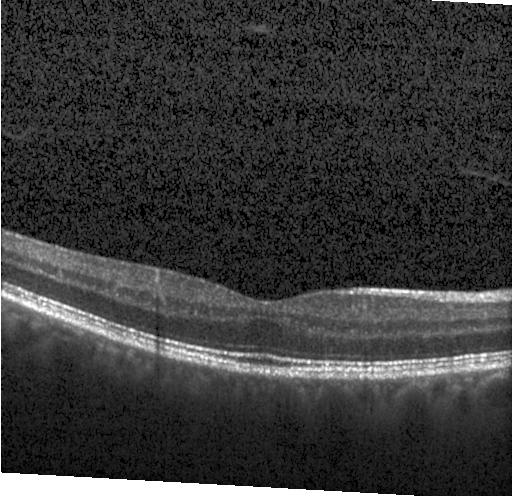
Heidelberg Spectralis · SD-OCT · OCT line scan · macular scan
Finding: no CNV, no DME, and no drusen.